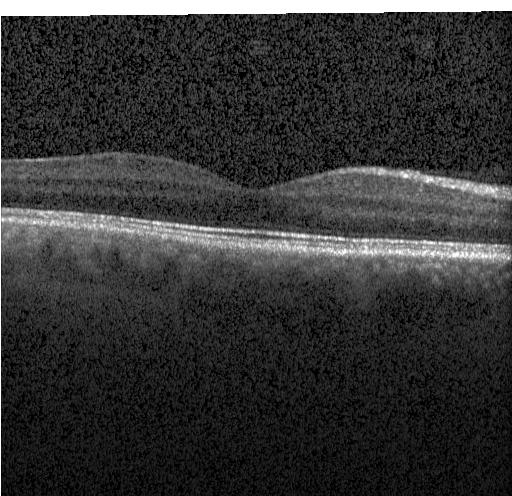 Optical coherence tomography B-scan
This B-scan demonstrates no CNV, no DME, and no drusen.